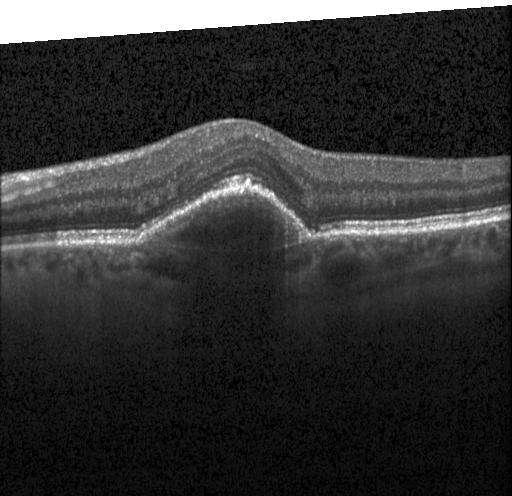
Spectral-domain optical coherence tomography. Heidelberg Spectralis. OCT B-scan — This B-scan demonstrates a choroidal neovascular membrane.